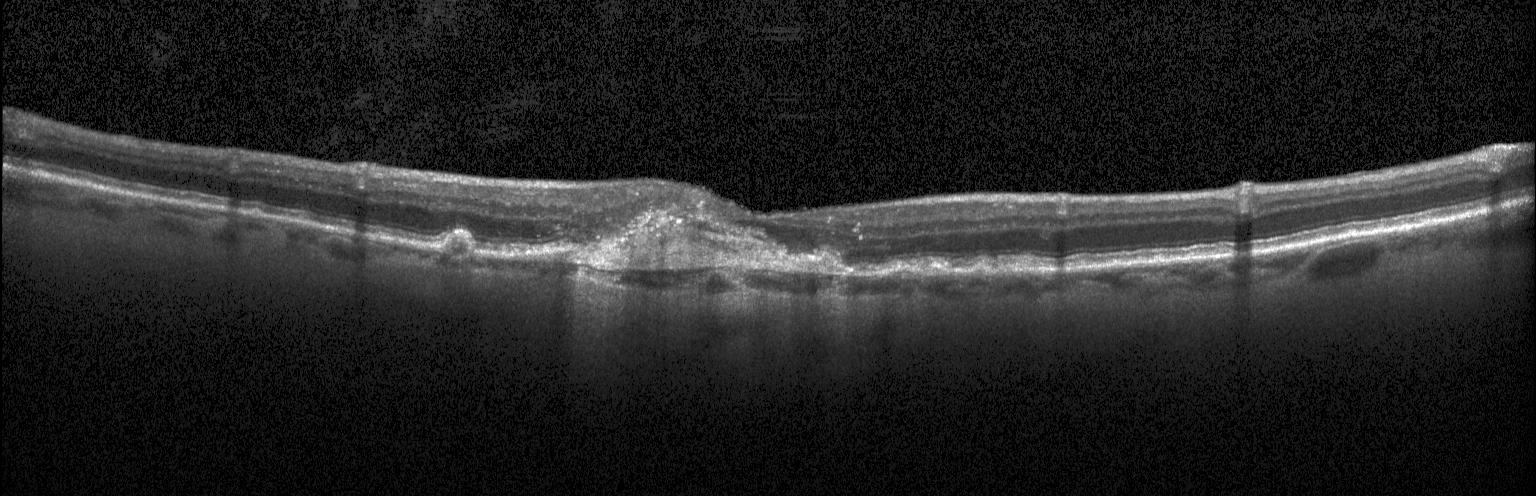

Dx: a choroidal neovascular membrane.